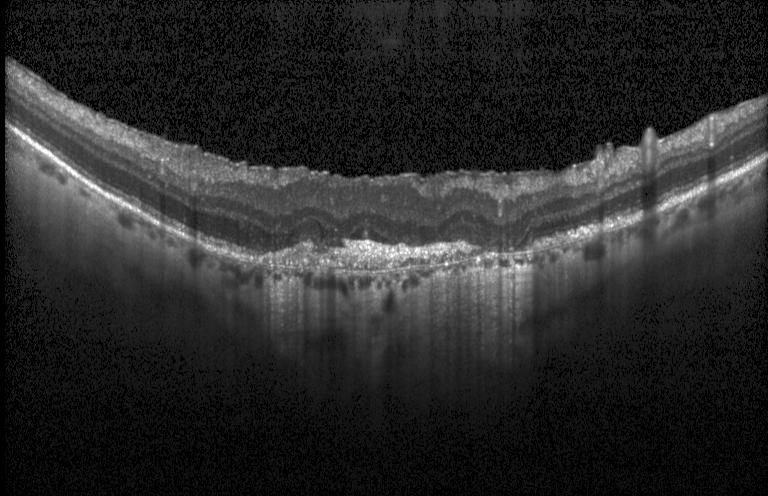 OCT B-scan; macular scan; spectral-domain OCT — Diagnosis: a choroidal neovascular membrane.